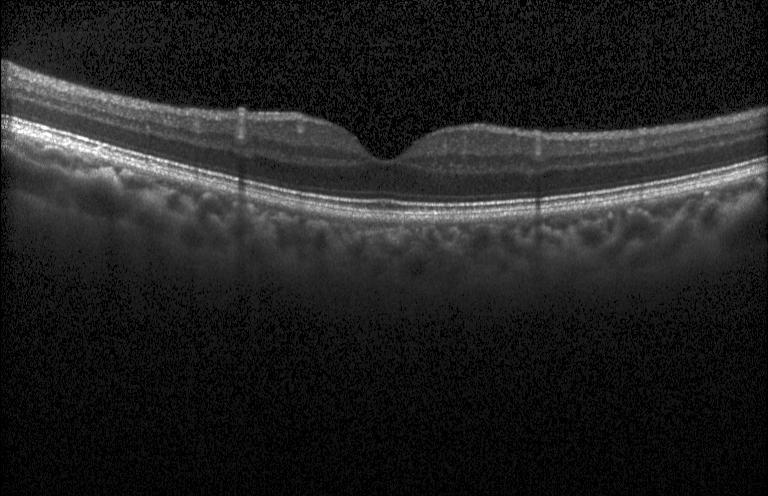
Spectral-domain optical coherence tomography; retinal OCT B-scan
This B-scan demonstrates no evidence of choroidal neovascularization, diabetic macular edema, or drusen.